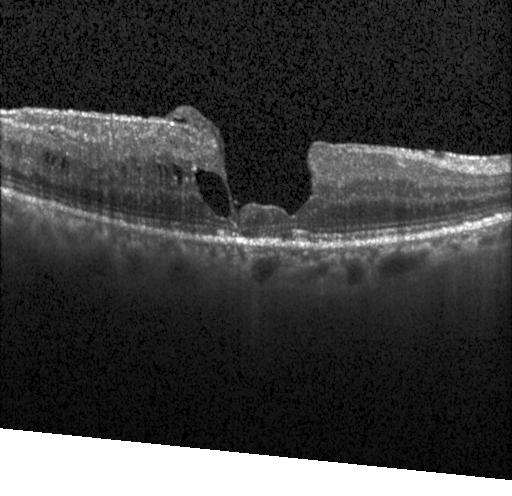 Retinal OCT cross-section. SD-OCT. Heidelberg Spectralis
Macular OCT: DME.